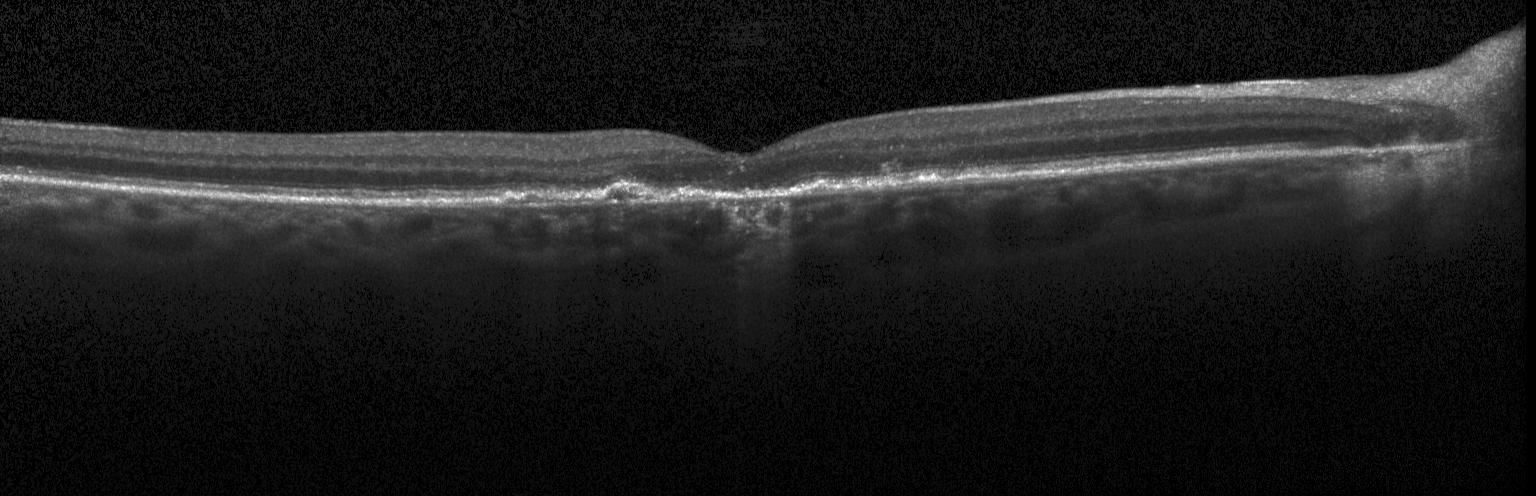 Instrument: Heidelberg Spectralis · retinal OCT B-scan · SD-OCT · horizontal scan through the fovea. Diagnosis: a choroidal neovascular membrane.